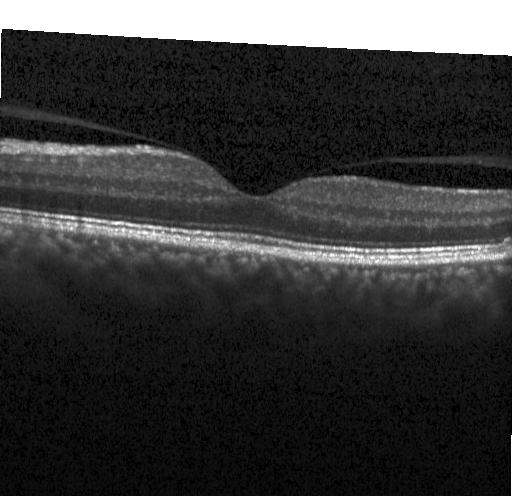

No choroidal neovascularization, no diabetic macular edema, and no drusen.